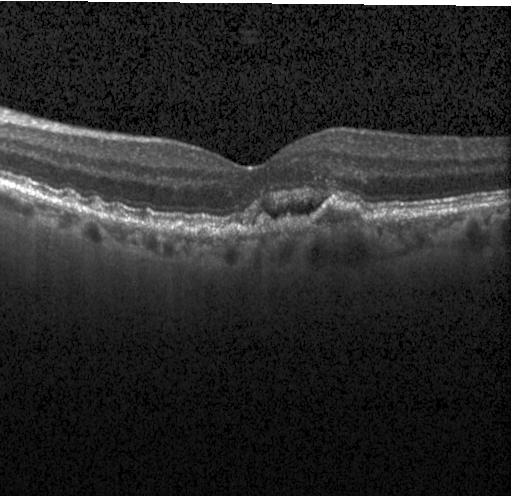

A choroidal neovascular membrane.